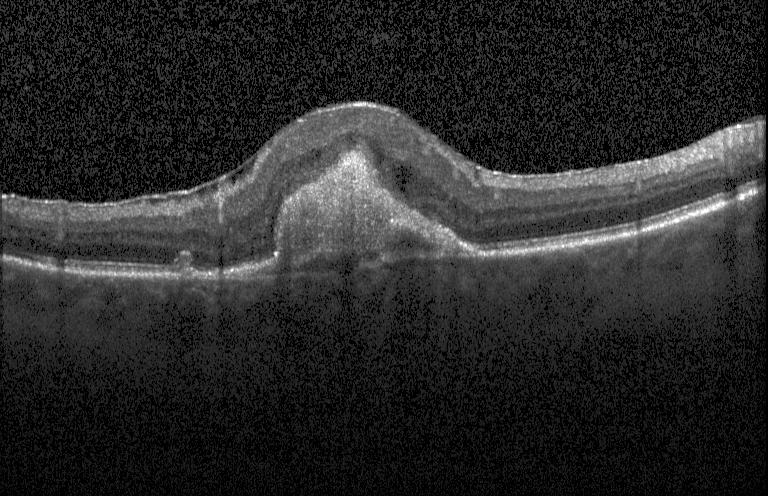
This B-scan demonstrates choroidal neovascularization.